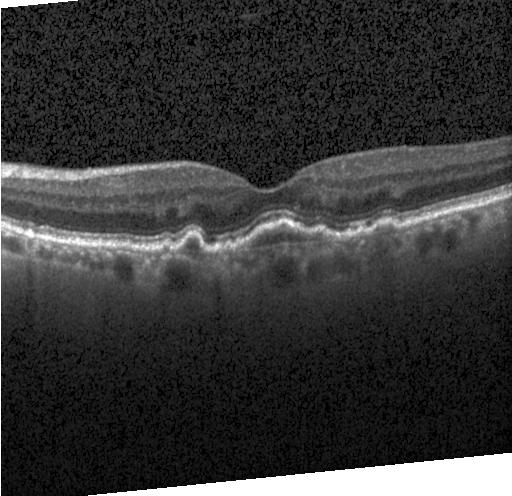
OCT line scan — Assessment: CNV.